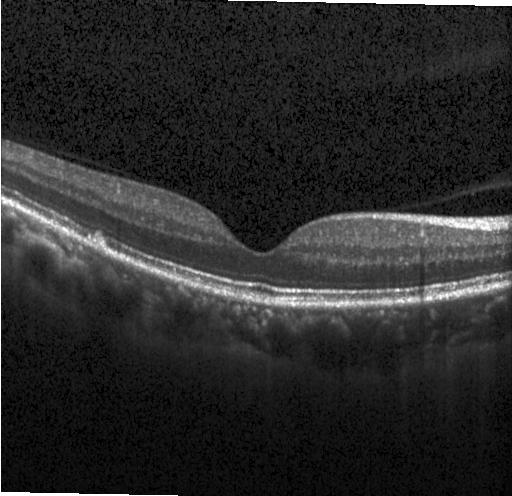

Heidelberg Spectralis OCT system. Retinal OCT B-scan.
Impression: drusen.